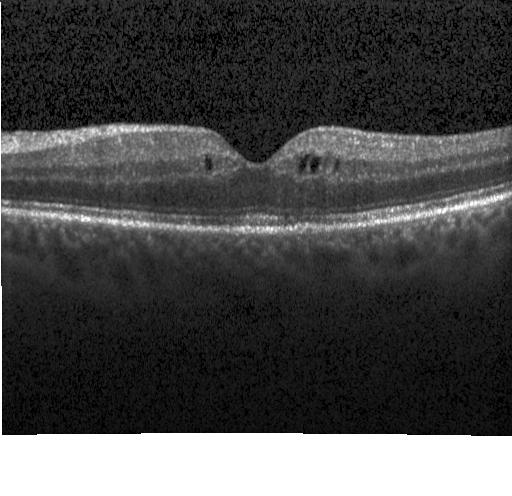 Retinal OCT cross-section. Spectral-domain optical coherence tomography. Heidelberg Spectralis. Fovea-centered. Diagnosis: diabetic macular edema (DME).